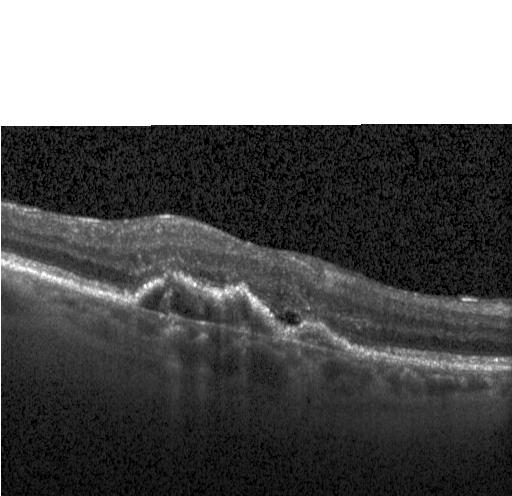

Spectral-domain OCT, centered on the fovea, OCT line scan, Heidelberg Spectralis OCT system. Dx: CNV.